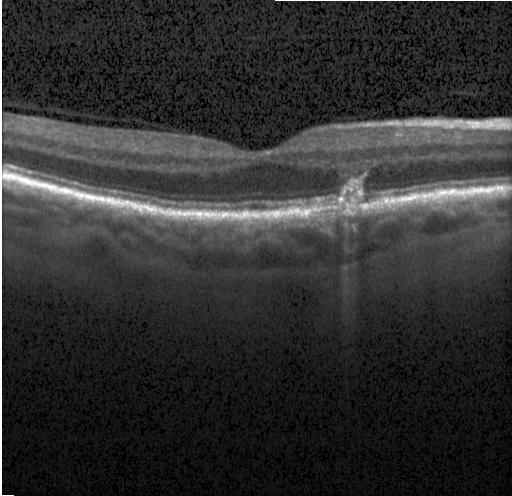

Centered on the fovea · spectral-domain OCT · instrument: Heidelberg Spectralis · OCT B-scan — This B-scan demonstrates drusen.